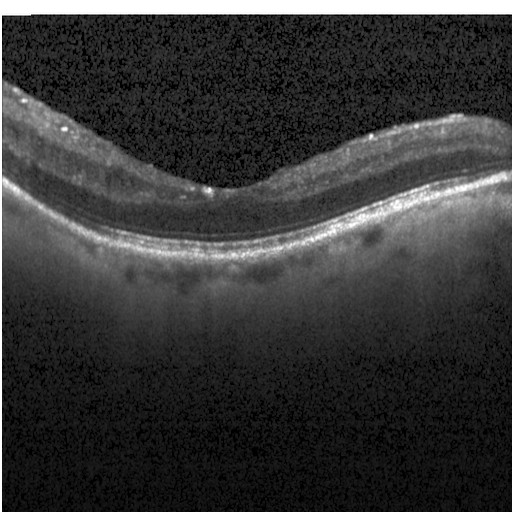

Optical coherence tomography scan
The scan shows diabetic macular edema (DME).